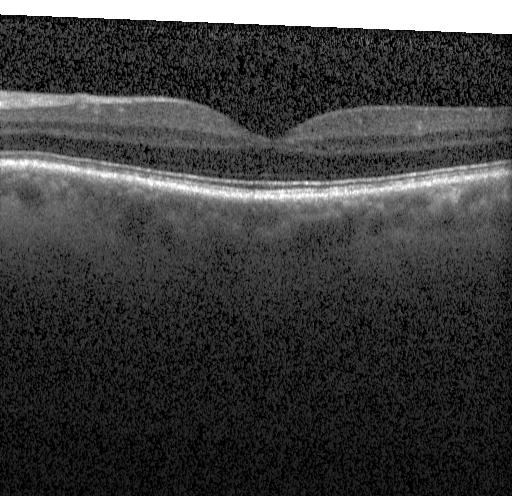
SD-OCT, centered on the fovea, retinal OCT B-scan.
Diagnosis: no choroidal neovascularization, no diabetic macular edema, and no drusen.